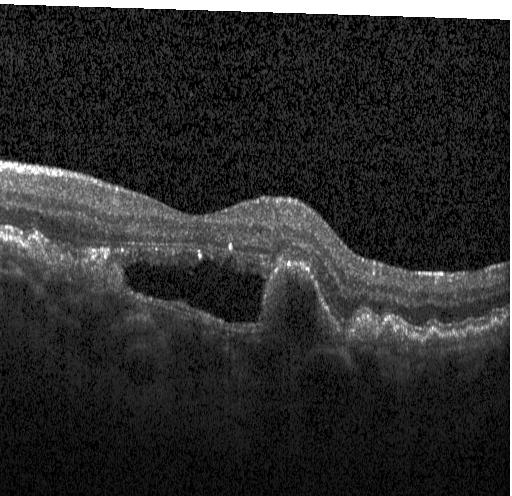

Optical coherence tomography B-scan. Macular scan
OCT finding: a choroidal neovascular membrane.